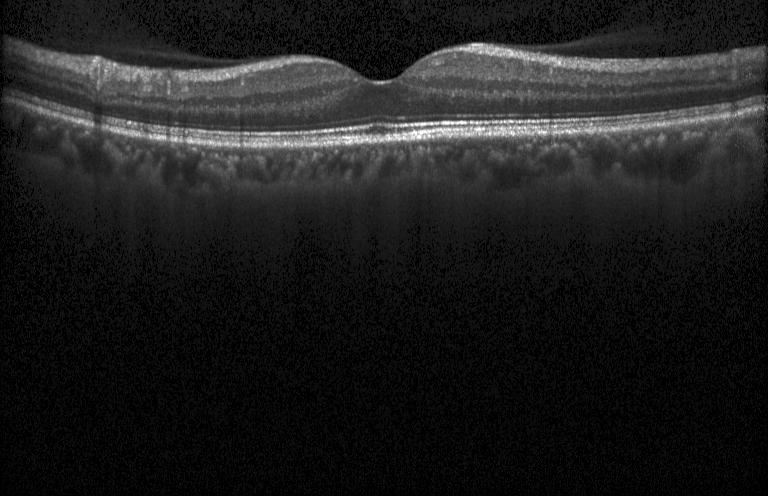
Spectral-domain OCT; retinal OCT cross-section; instrument: Heidelberg Spectralis; macular scan. Impression: no evidence of CNV, DME, or drusen.